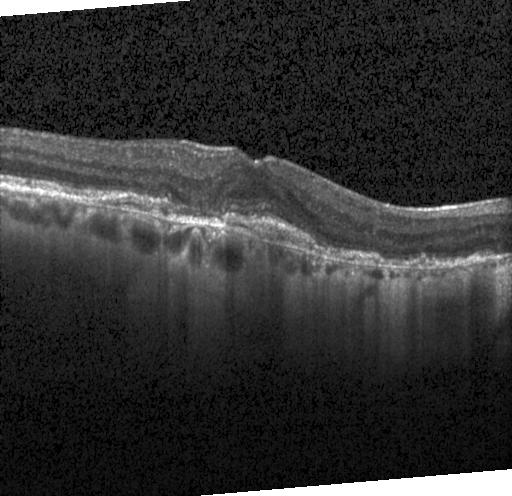 Spectral-domain optical coherence tomography, macular scan, optical coherence tomography scan — Dx: choroidal neovascularization.